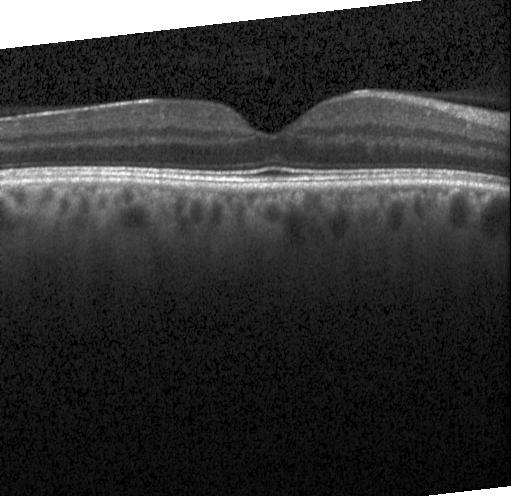
Spectral-domain optical coherence tomography; optical coherence tomography scan; horizontal scan through the fovea.
Impression: no choroidal neovascularization, no diabetic macular edema, and no drusen.